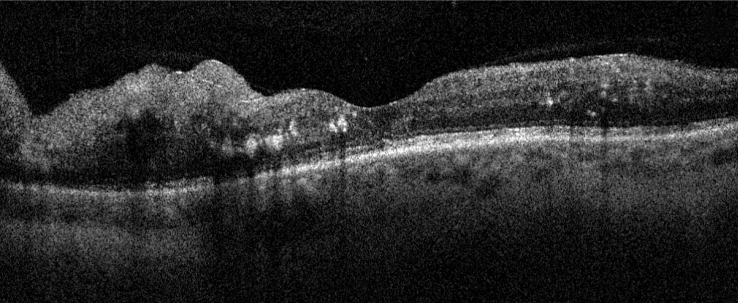 Acquired on an Optovue Avanti RTVue XR · through the macula · optical coherence tomography scan — The scan shows diabetic macular edema.